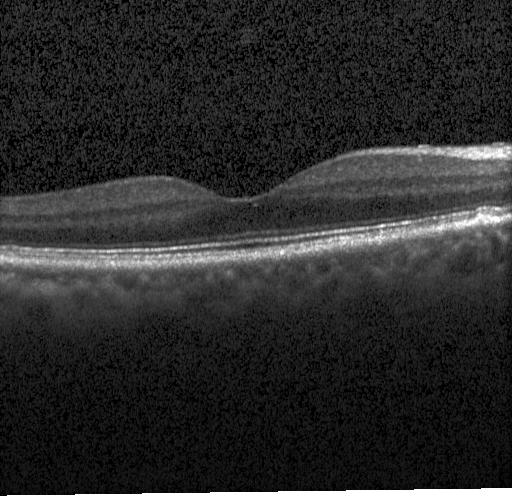
Retinal OCT B-scan
Macular OCT: no CNV, DME, or drusen.